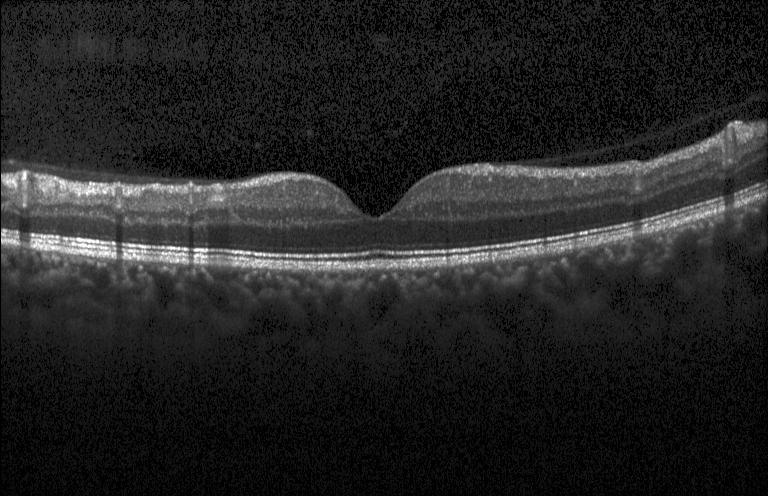
Through the macula; retinal OCT B-scan; spectral-domain optical coherence tomography. This B-scan demonstrates no choroidal neovascularization, diabetic macular edema, or drusen.